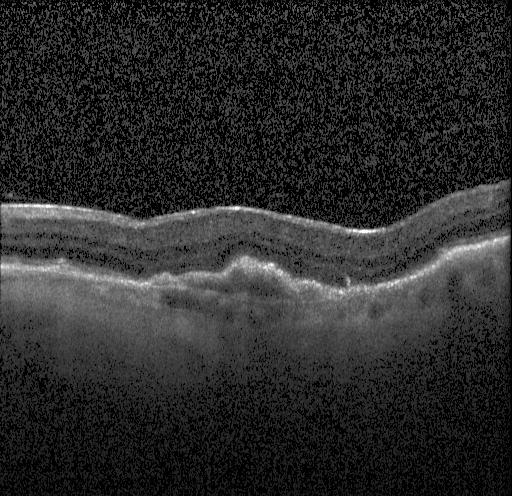
Optical coherence tomography B-scan
Finding: choroidal neovascularization.